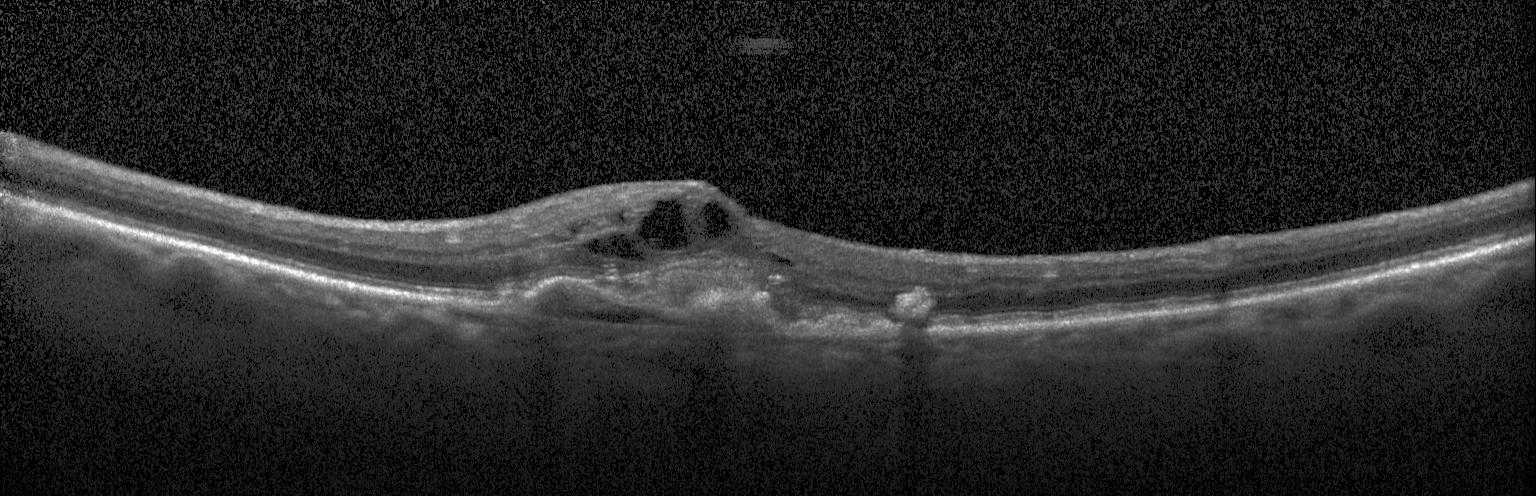
Impression: a choroidal neovascular membrane.